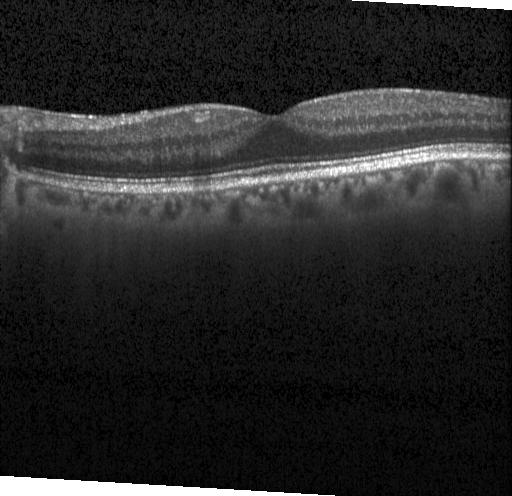

Retinal OCT cross-section, Heidelberg Spectralis — Diagnosis: neither choroidal neovascularization, diabetic macular edema, nor drusen.